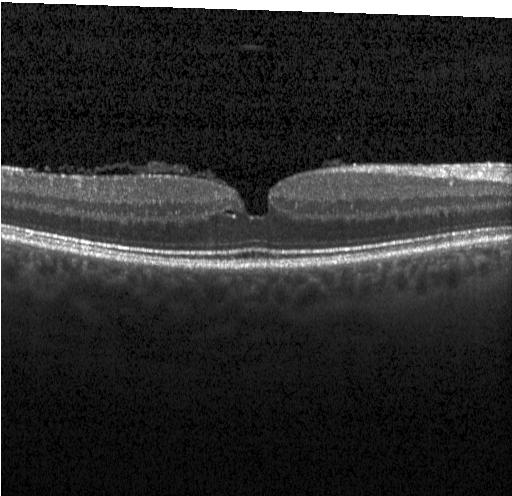 OCT B-scan.
OCT finding: diabetic macular edema.